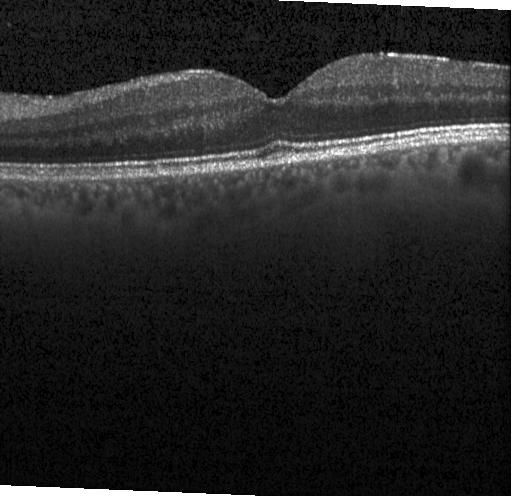 Retinal OCT cross-section
Finding: no choroidal neovascularization, no diabetic macular edema, and no drusen.